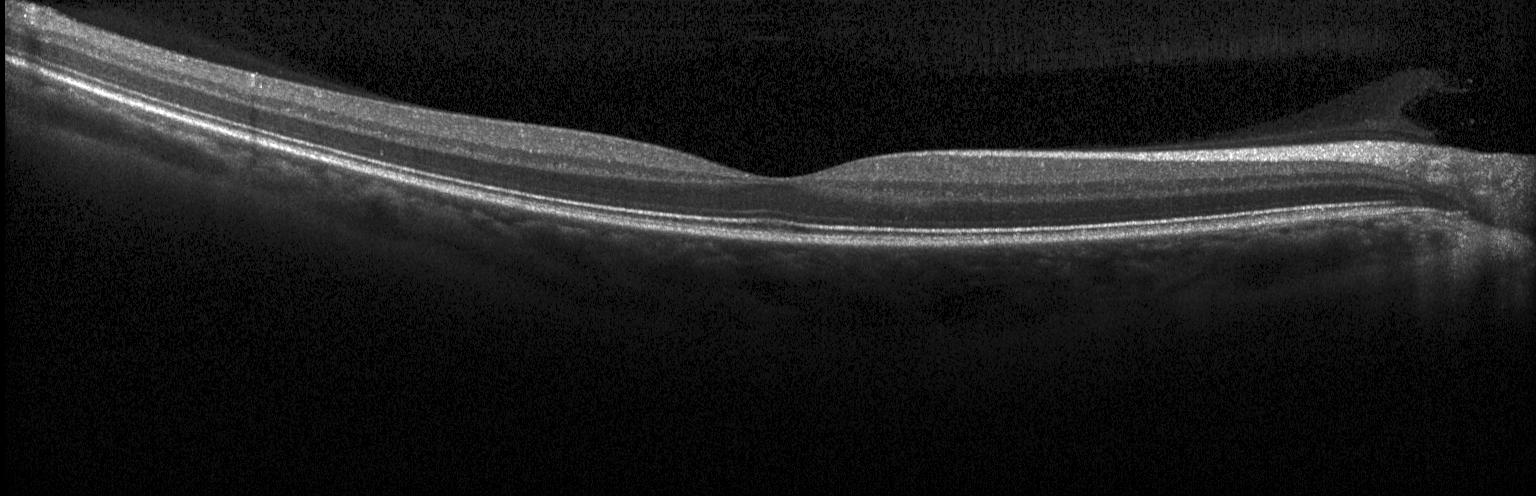
SD-OCT. Fovea-centered. Optical coherence tomography B-scan. Acquired on a Heidelberg Spectralis
OCT finding: no CNV, DME, or drusen.